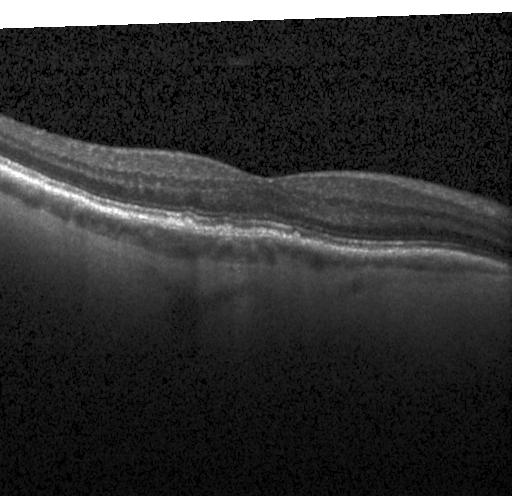
Acquired on a Heidelberg Spectralis, retinal OCT cross-section. Finding: multiple drusen.